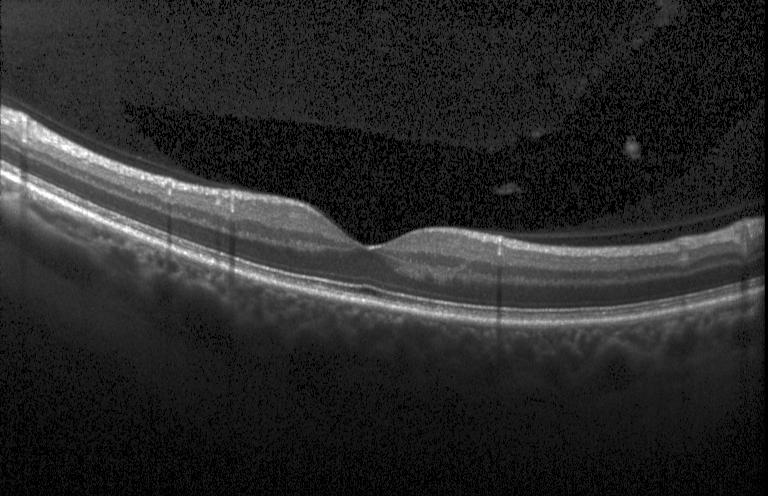
Spectral-domain optical coherence tomography; retinal OCT B-scan; instrument: Heidelberg Spectralis
Macular OCT: no evidence of choroidal neovascularization, diabetic macular edema, or drusen.